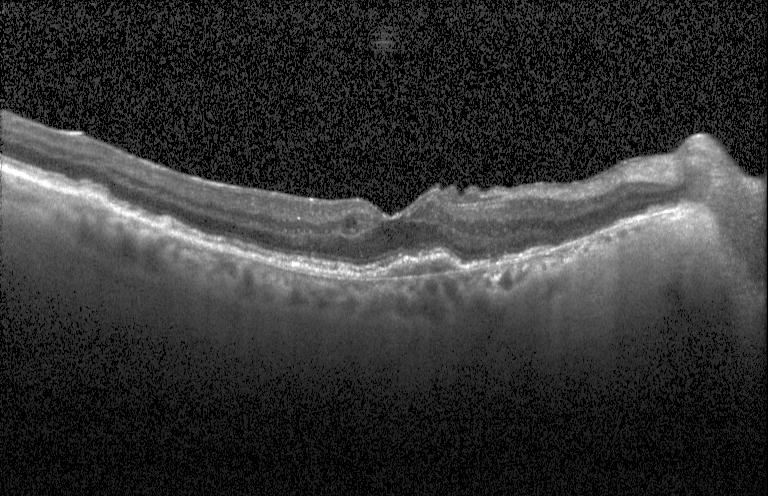
OCT line scan, horizontal scan through the fovea
Macular OCT: a choroidal neovascular membrane.